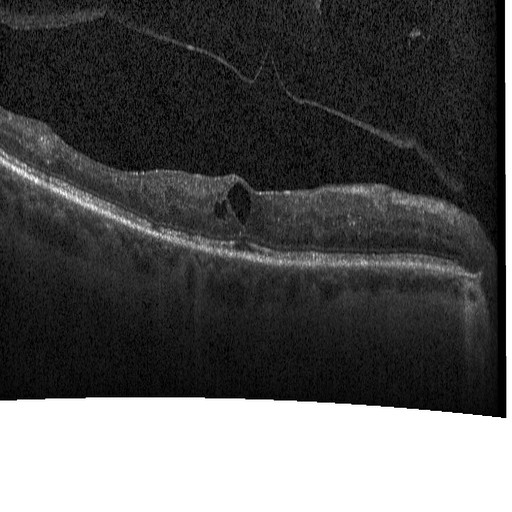

Spectral-domain optical coherence tomography; OCT B-scan. This B-scan demonstrates diabetic macular edema.